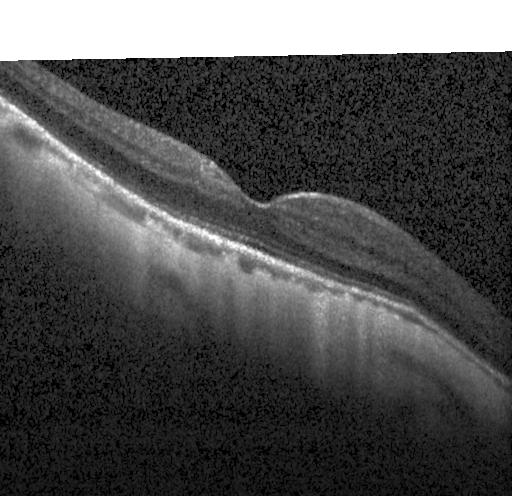
OCT finding: no CNV, DME, or drusen.